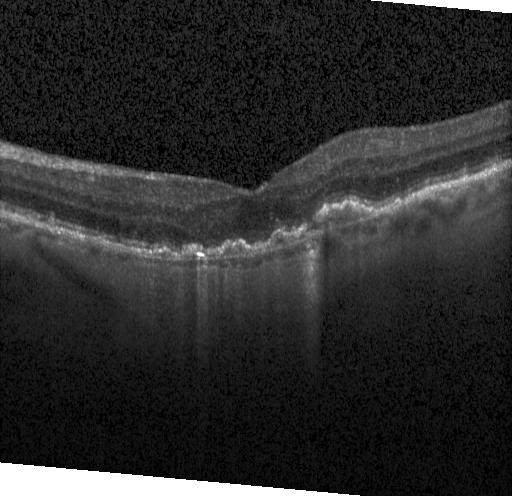
Retinal OCT cross-section.
This B-scan demonstrates a choroidal neovascular membrane.